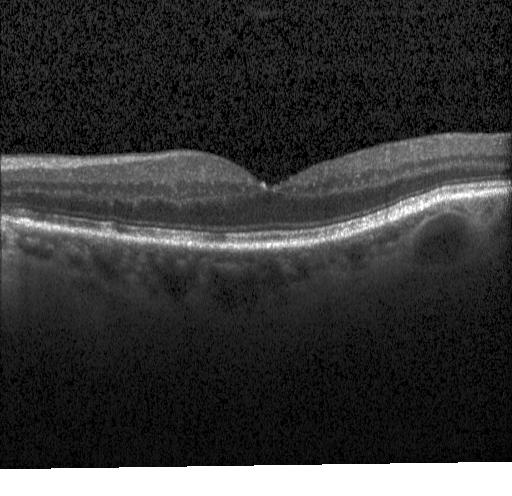

Impression: no evidence of choroidal neovascularization, diabetic macular edema, or drusen.